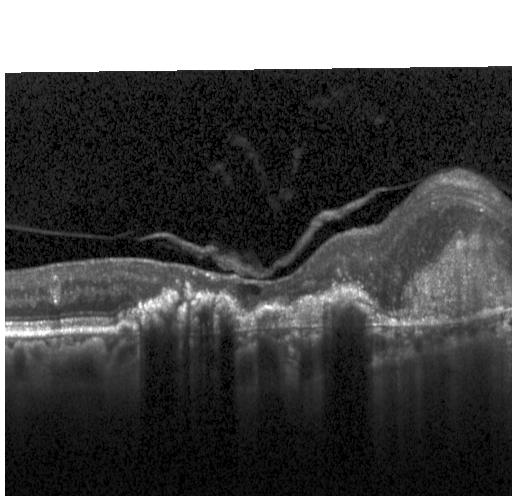
Optical coherence tomography scan — Assessment: a choroidal neovascular membrane.